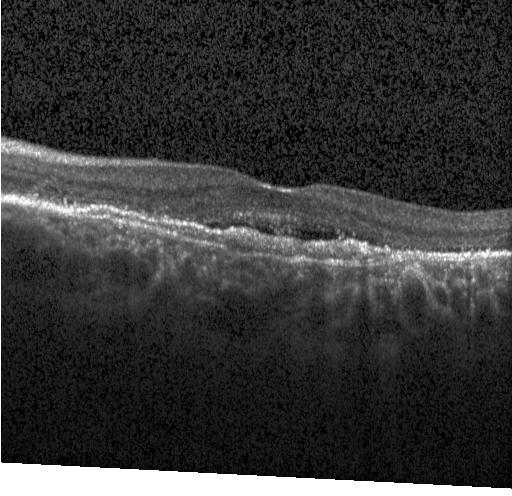 Horizontal scan through the fovea, Heidelberg Spectralis, optical coherence tomography scan. Macular OCT: choroidal neovascularization (CNV).